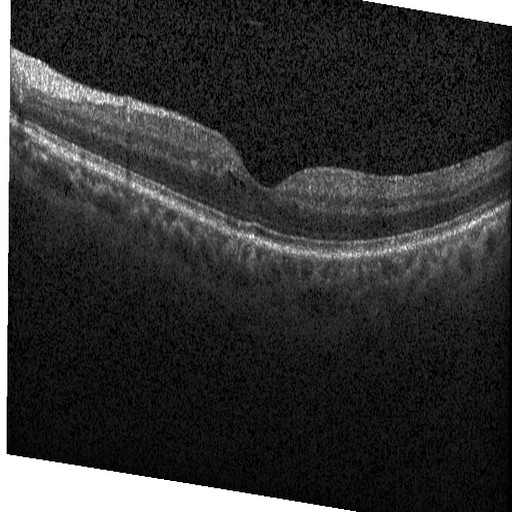
Diagnosis: DME.